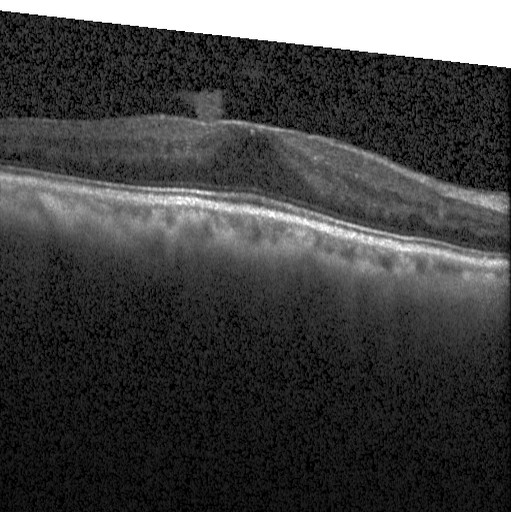 Retinal OCT B-scan · macular scan. OCT finding: diabetic macular edema (DME).